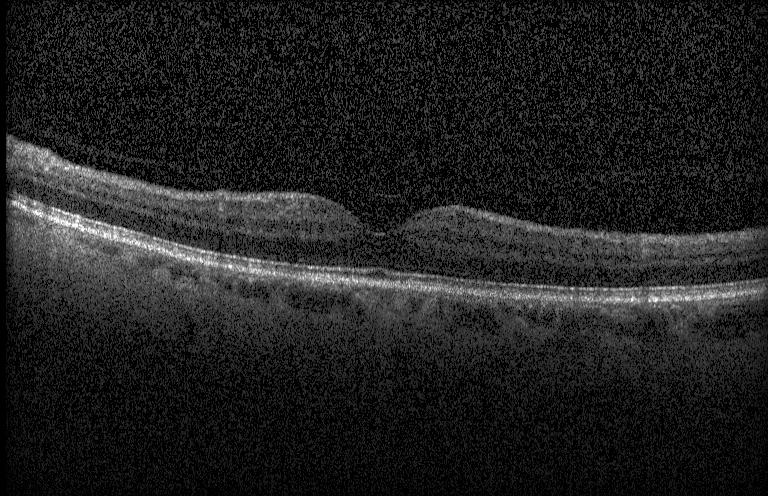 OCT B-scan.
Assessment: neither choroidal neovascularization, diabetic macular edema, nor drusen.